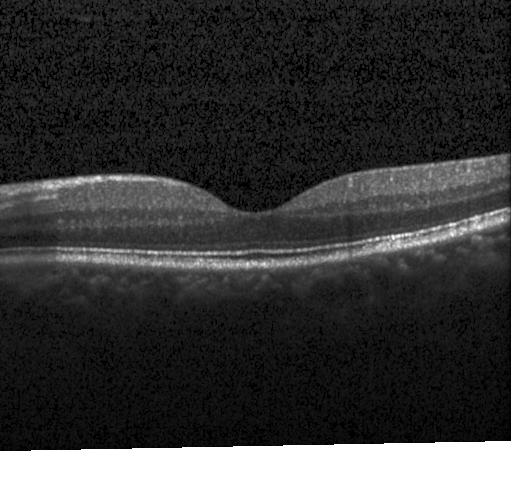 Through the macula, Heidelberg Spectralis, optical coherence tomography B-scan.
Assessment: no CNV, DME, or drusen.